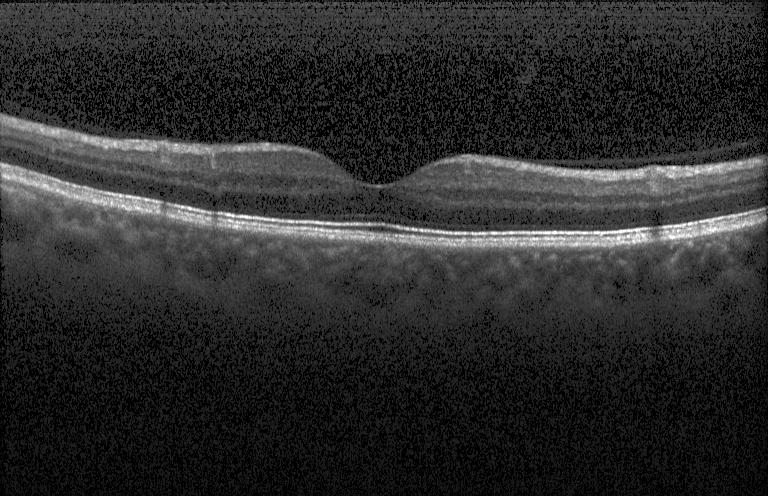

Optical coherence tomography scan.
This B-scan demonstrates no choroidal neovascularization, no diabetic macular edema, and no drusen.